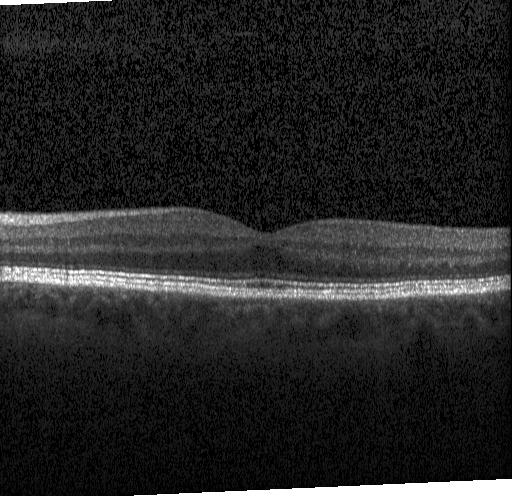

OCT B-scan · spectral-domain optical coherence tomography.
Assessment: no CNV, no DME, and no drusen.